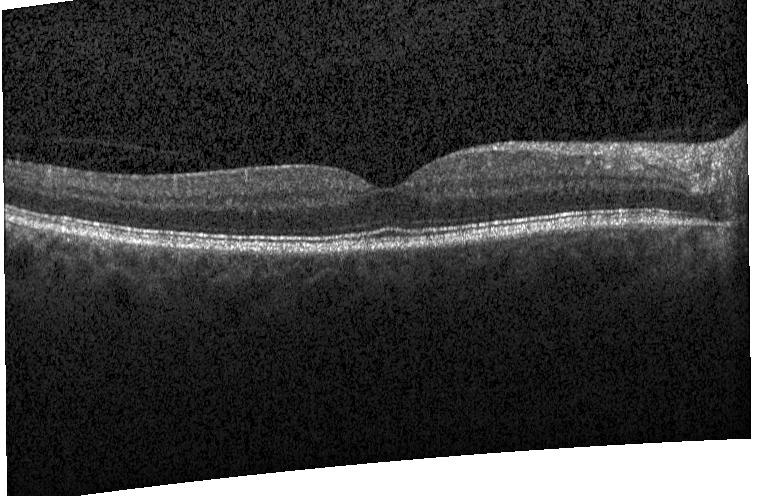 Spectral-domain OCT. Optical coherence tomography B-scan. Through the macula. Heidelberg Spectralis OCT system — Diagnosis: neither choroidal neovascularization, diabetic macular edema, nor drusen.